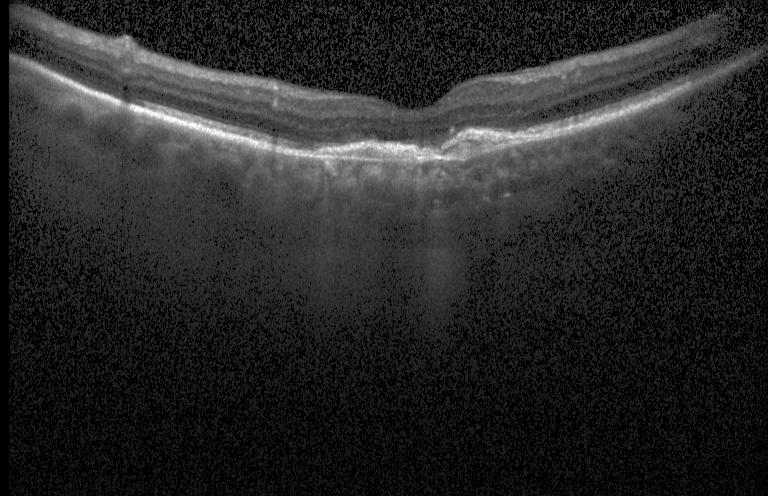
Macular OCT: CNV.